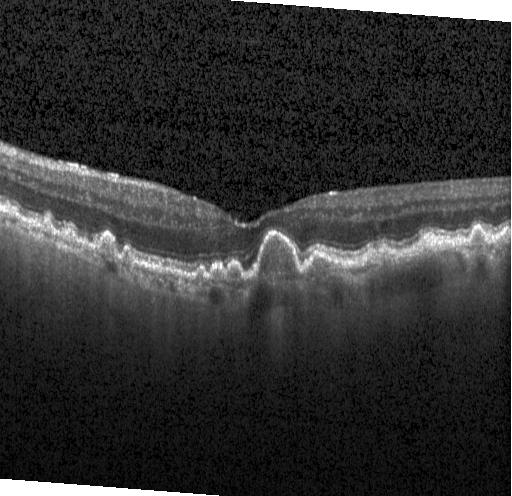
OCT B-scan showing sub-RPE drusenoid deposits.